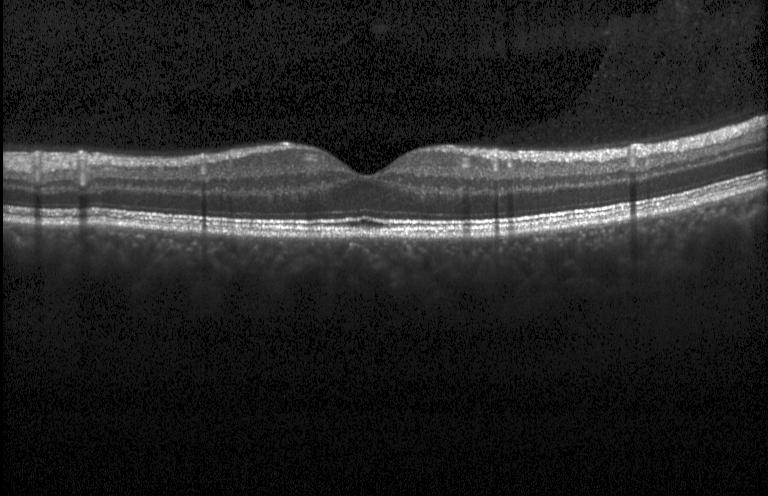
OCT B-scan
Diagnosis: no choroidal neovascularization, no diabetic macular edema, and no drusen.